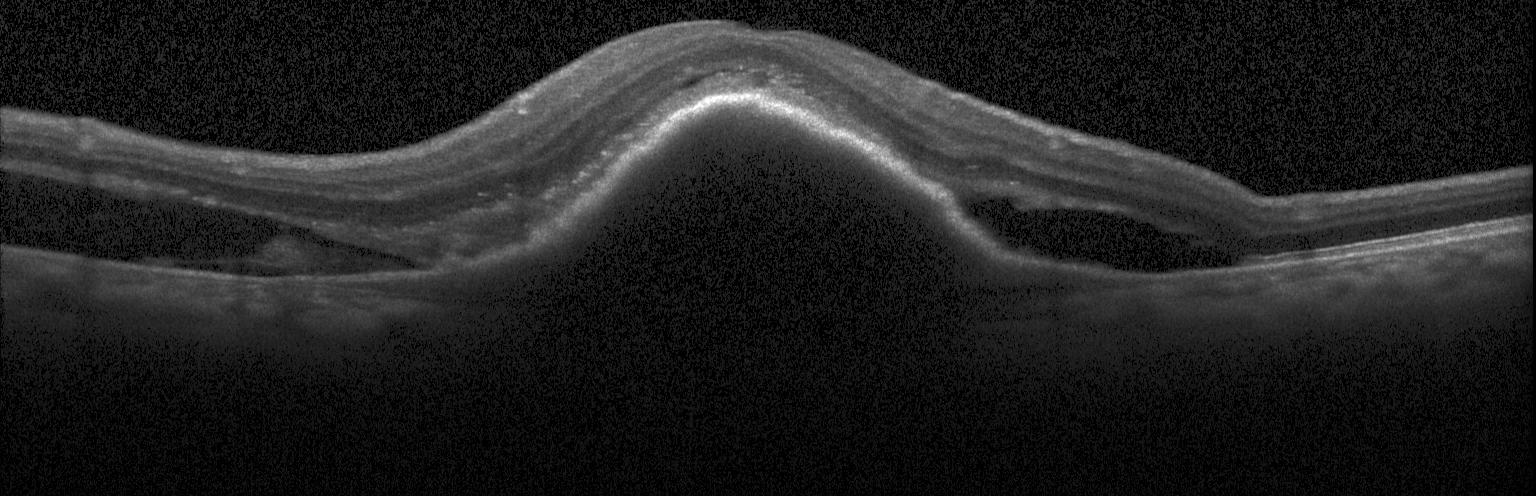
Optical coherence tomography B-scan · acquired on a Heidelberg Spectralis
OCT finding: a choroidal neovascular membrane.